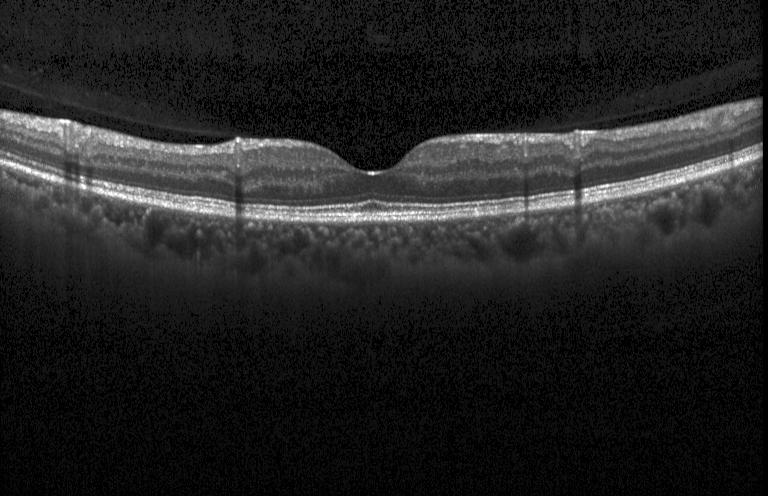

Optical coherence tomography scan
Impression: no evidence of CNV, DME, or drusen.